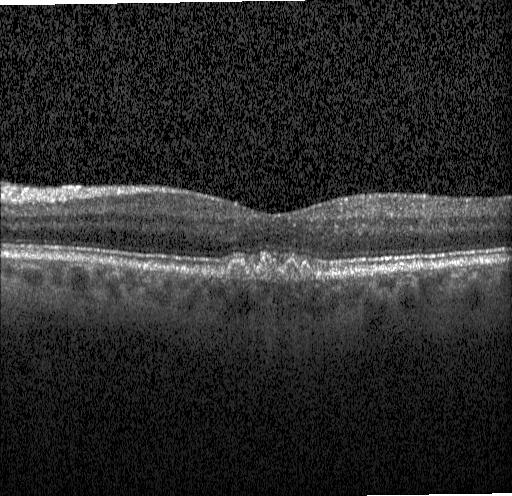

OCT B-scan · acquired on a Heidelberg Spectralis.
The scan shows drusen.